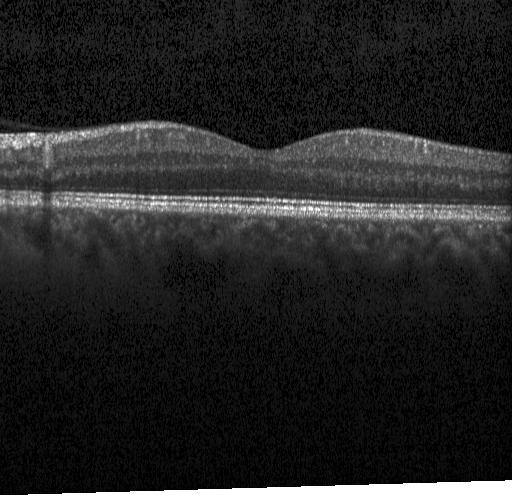
Acquired on a Heidelberg Spectralis, fovea-centered, spectral-domain OCT, retinal OCT B-scan. The scan shows neither choroidal neovascularization, diabetic macular edema, nor drusen.